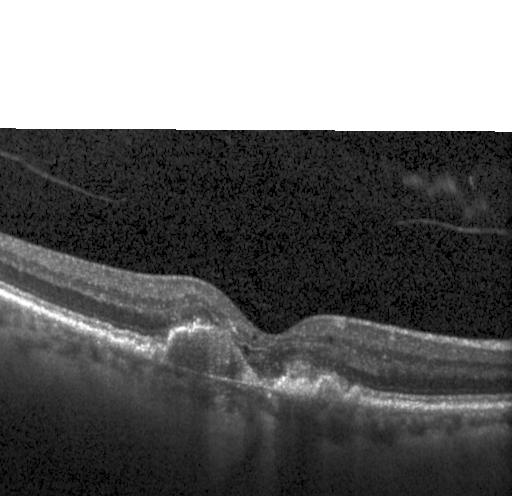

Retinal OCT cross-section. Finding: choroidal neovascularization.